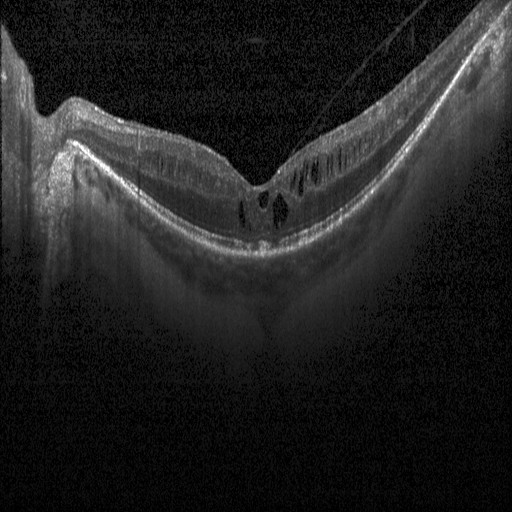 OCT B-scan; fovea-centered; Heidelberg Spectralis; spectral-domain optical coherence tomography
DME.